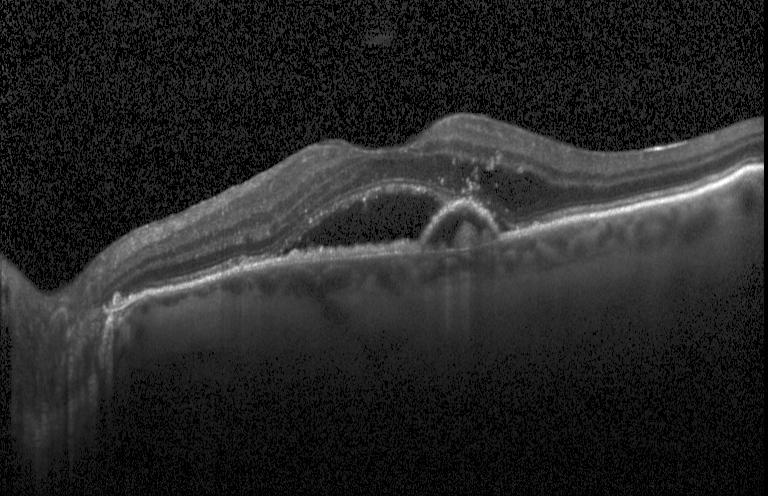 OCT B-scan
OCT finding: a choroidal neovascular membrane.